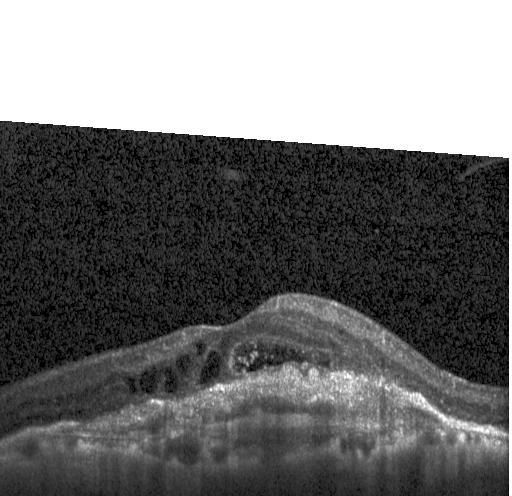

OCT finding: a choroidal neovascular membrane.